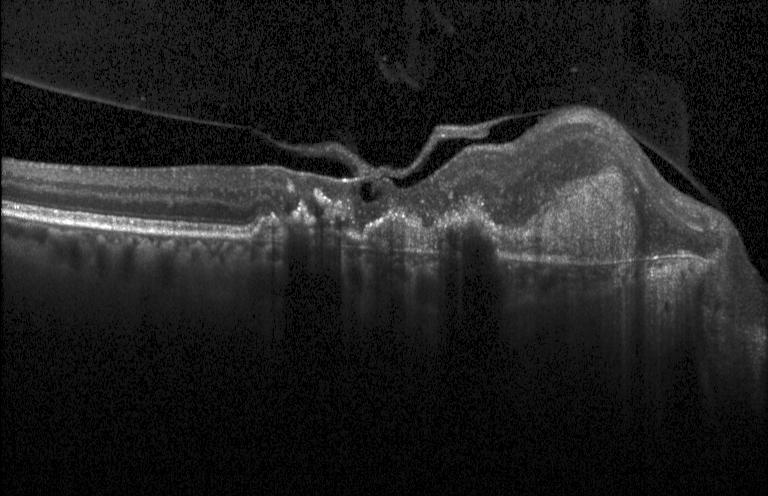
Spectral-domain OCT. Optical coherence tomography scan. Heidelberg Spectralis. Fovea-centered
The scan shows CNV.